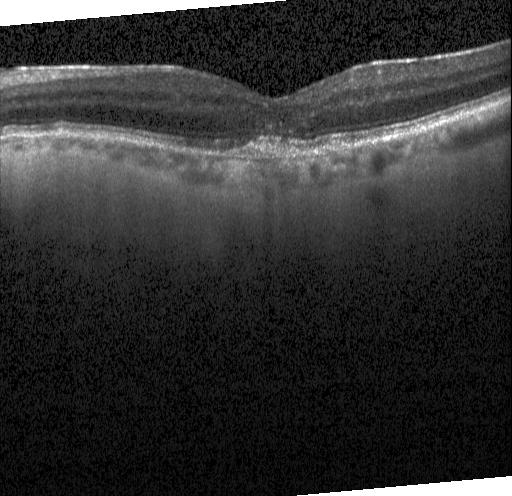 Impression: choroidal neovascularization.